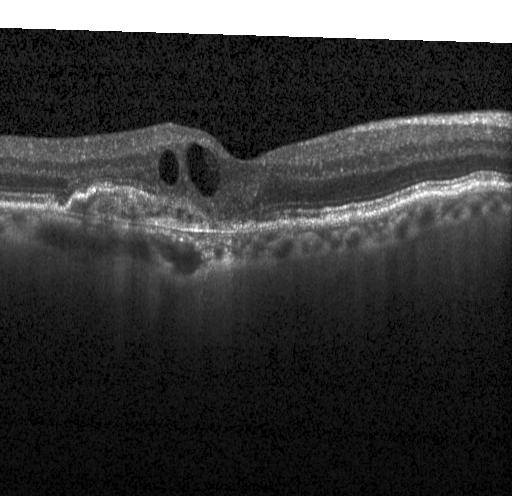
Instrument: Heidelberg Spectralis. Optical coherence tomography scan. Spectral-domain OCT — Finding: choroidal neovascularization (CNV).